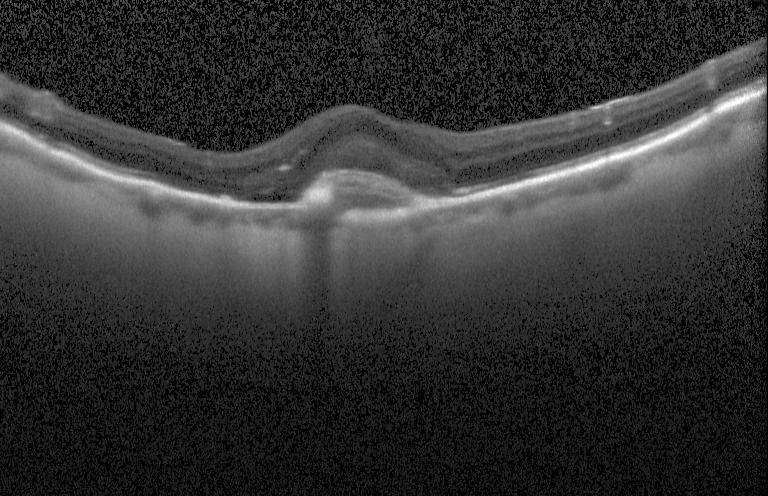

Macular OCT: a choroidal neovascular membrane.